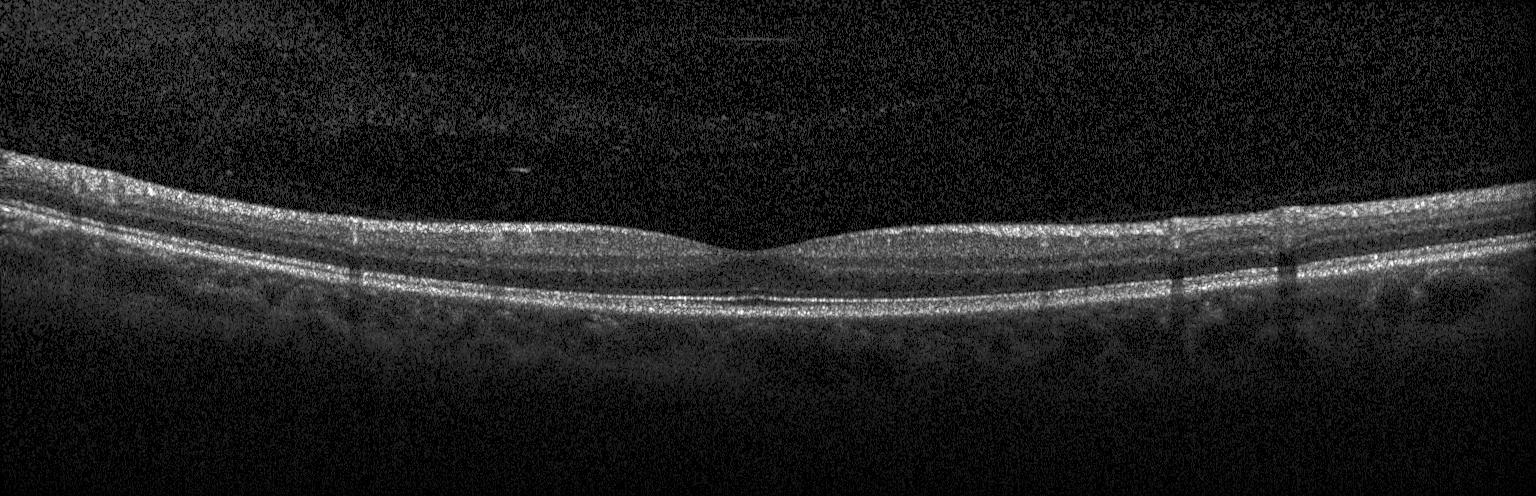
Impression: no choroidal neovascularization, no diabetic macular edema, and no drusen.